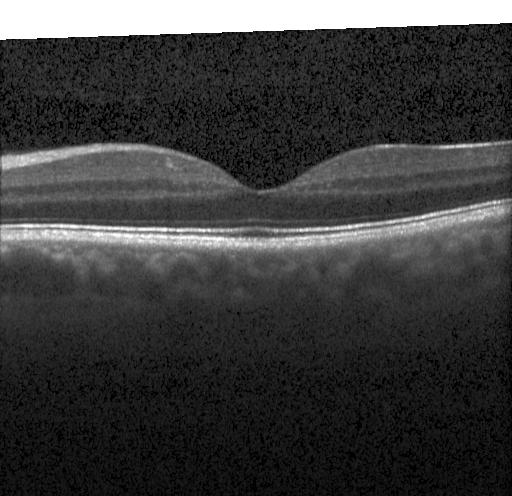 Dx: neither choroidal neovascularization, diabetic macular edema, nor drusen.